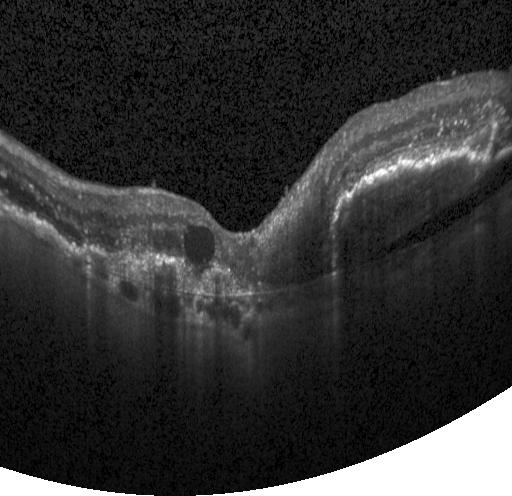 Retinal OCT cross-section, through the macula, spectral-domain OCT
OCT finding: a choroidal neovascular membrane.